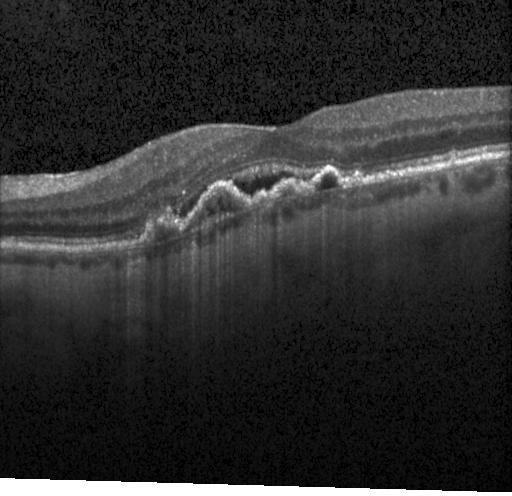

Retinal OCT B-scan; SD-OCT; instrument: Heidelberg Spectralis; macular scan.
Macular OCT: choroidal neovascularization.